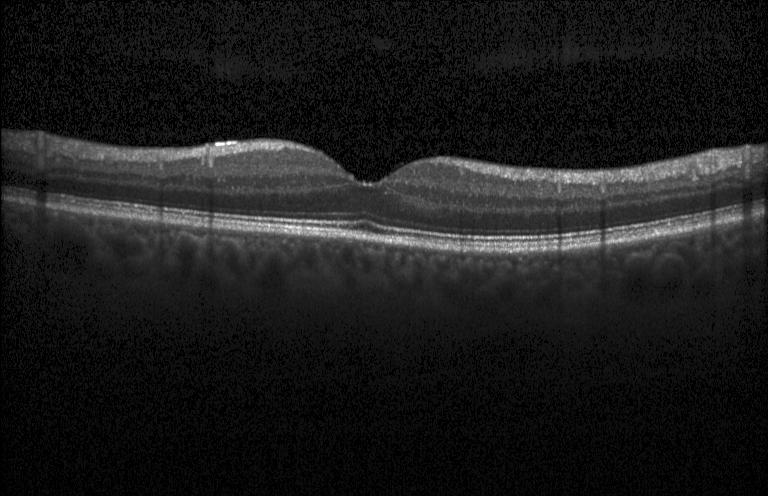
The scan shows neither choroidal neovascularization, diabetic macular edema, nor drusen.